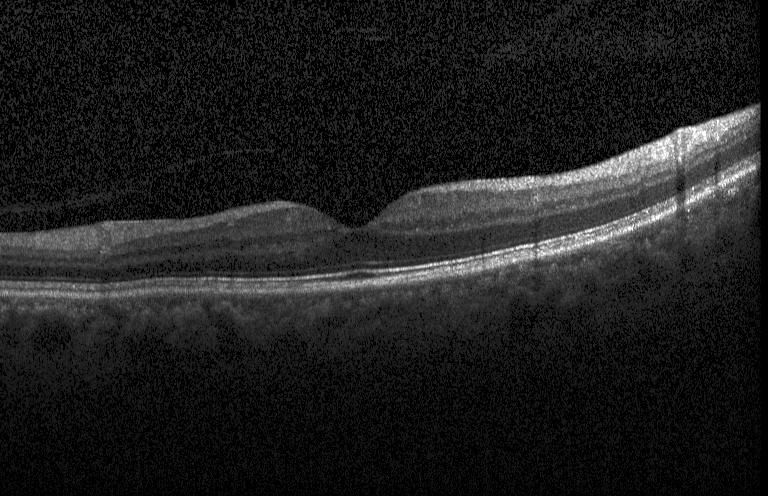

OCT line scan, spectral-domain OCT, centered on the fovea, instrument: Heidelberg Spectralis. The scan shows no CNV, DME, or drusen.